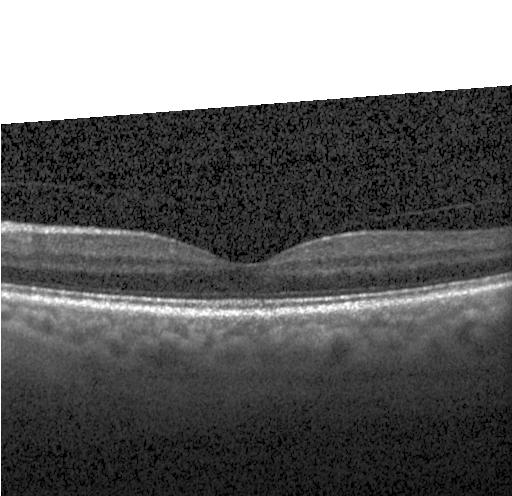
This B-scan demonstrates no choroidal neovascularization, diabetic macular edema, or drusen.